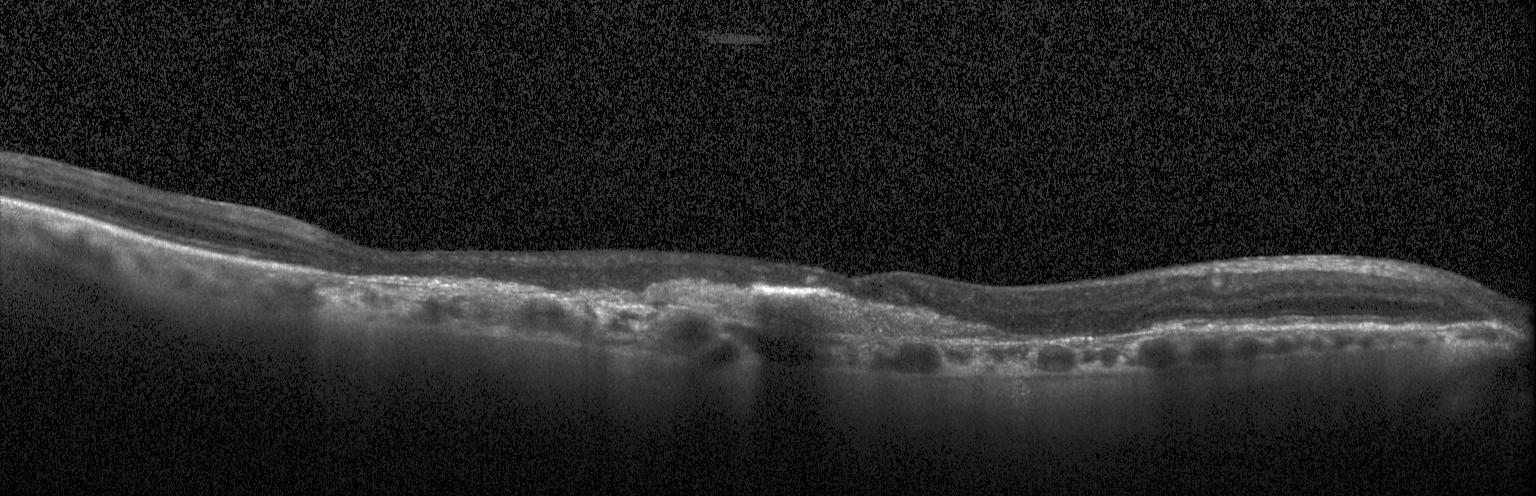
Macular scan, spectral-domain optical coherence tomography, retinal OCT cross-section — This B-scan demonstrates choroidal neovascularization.